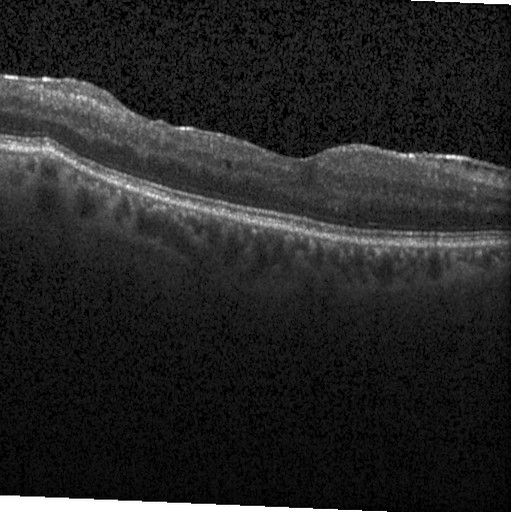

Horizontal scan through the fovea · spectral-domain OCT · Heidelberg Spectralis OCT system · OCT B-scan
OCT finding: DME.